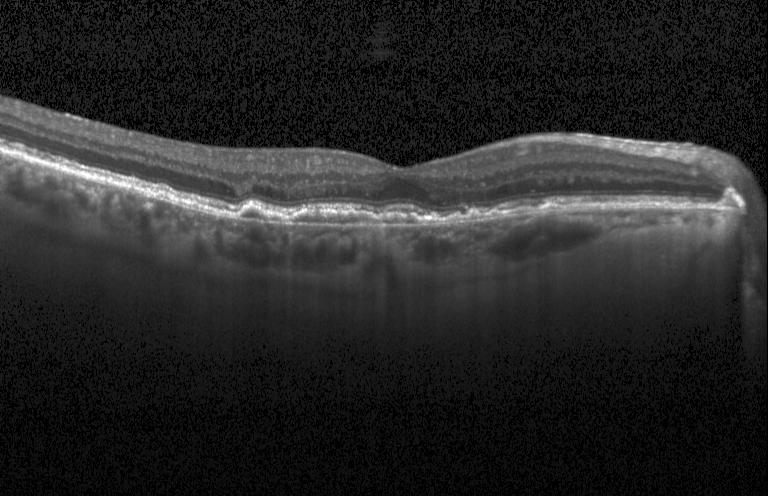
Retinal OCT cross-section, instrument: Heidelberg Spectralis, centered on the fovea, spectral-domain OCT
Impression: a choroidal neovascular membrane.